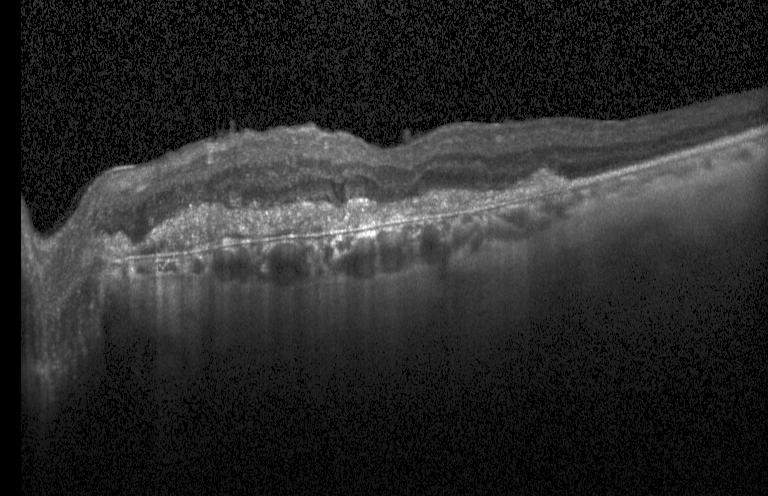
OCT scan showing a choroidal neovascular membrane.